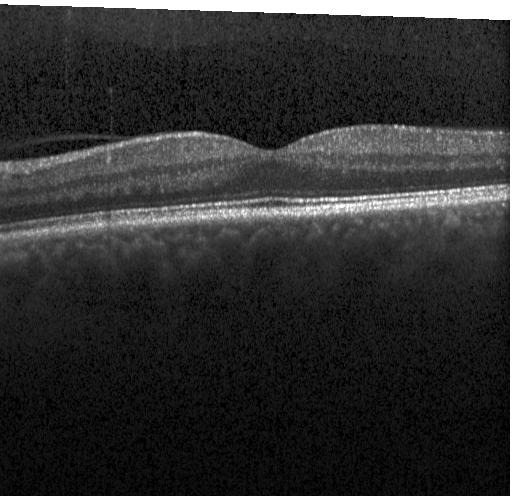

Optical coherence tomography B-scan. Macular OCT: no CNV, no DME, and no drusen.